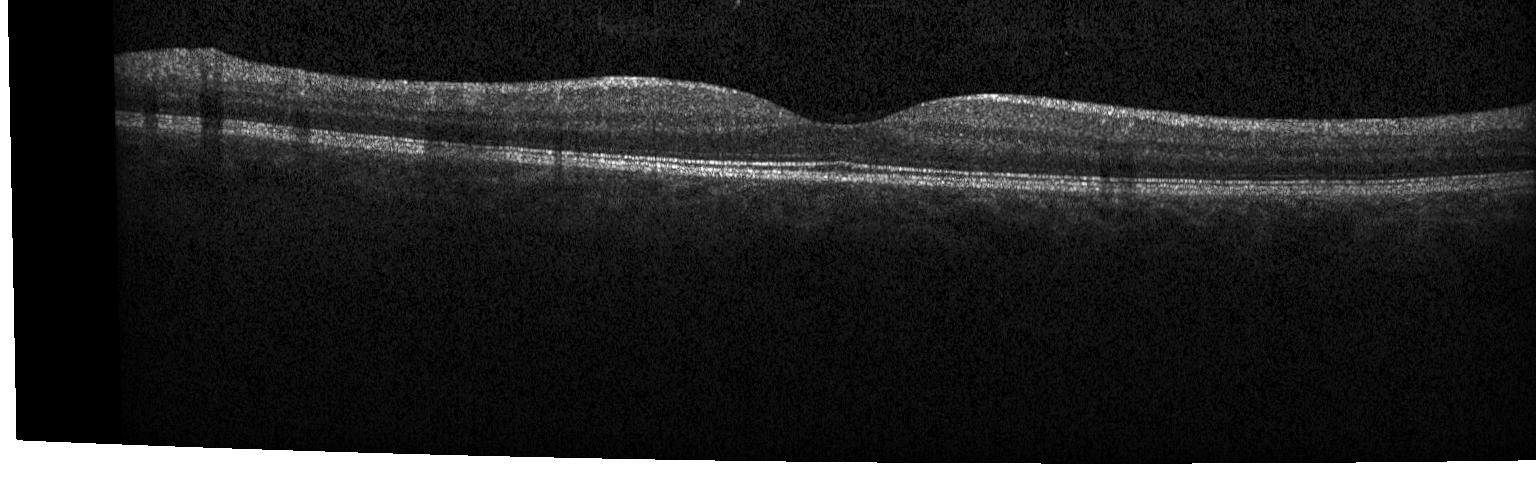

Fovea-centered, SD-OCT, retinal OCT B-scan, instrument: Heidelberg Spectralis. Finding: no choroidal neovascularization, no diabetic macular edema, and no drusen.